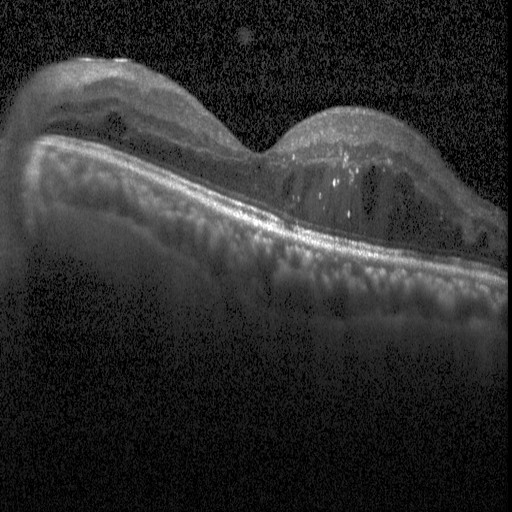 OCT B-scan.
Impression: diabetic macular edema (DME).